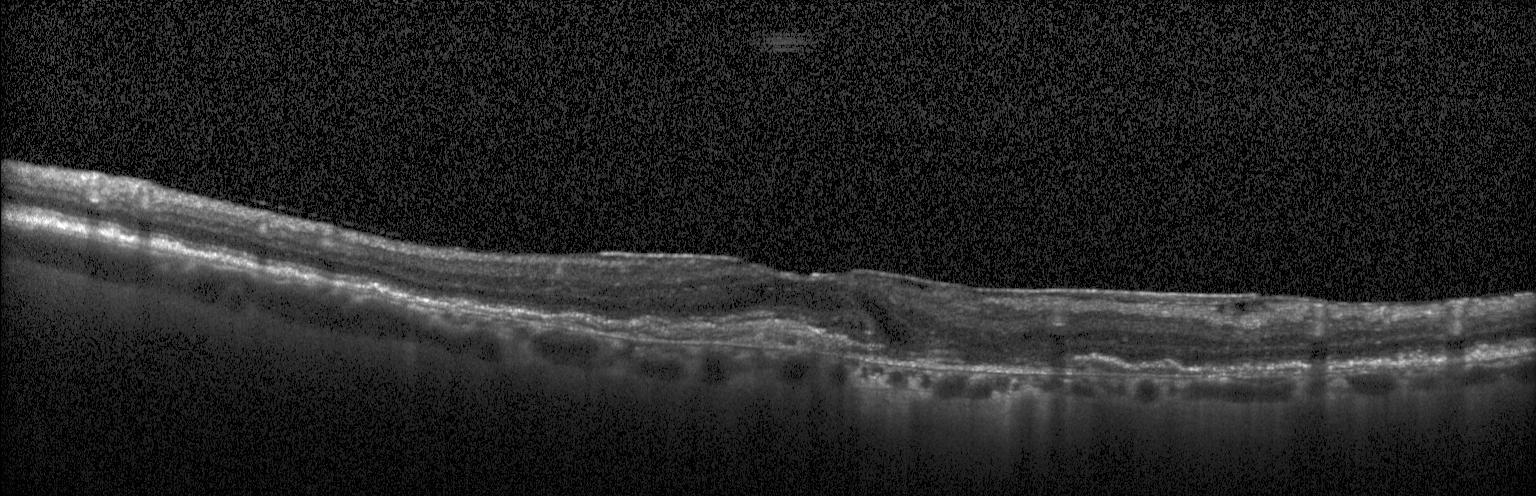

Optical coherence tomography B-scan; Heidelberg Spectralis OCT system — Finding: a choroidal neovascular membrane.